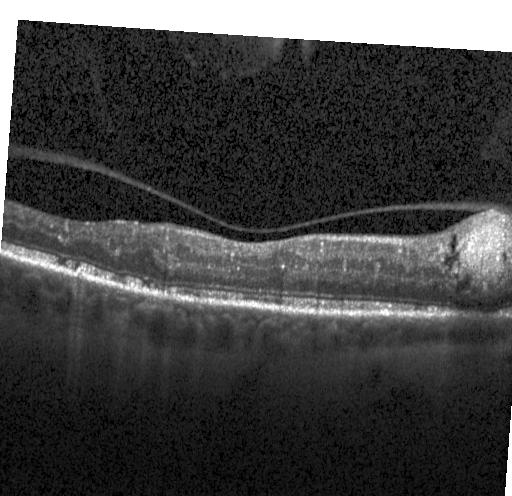
OCT B-scan — Impression: DME.